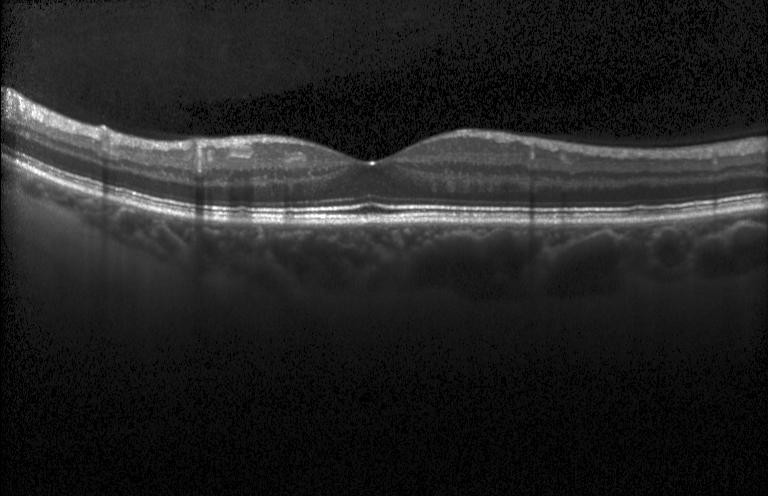
Macular OCT demonstrating no choroidal neovascularization, diabetic macular edema, or drusen.